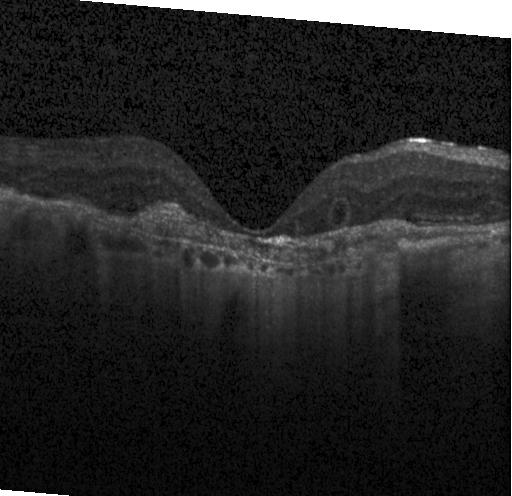
Acquired on a Heidelberg Spectralis. Spectral-domain OCT. Centered on the fovea. Optical coherence tomography B-scan — Dx: choroidal neovascularization (CNV).